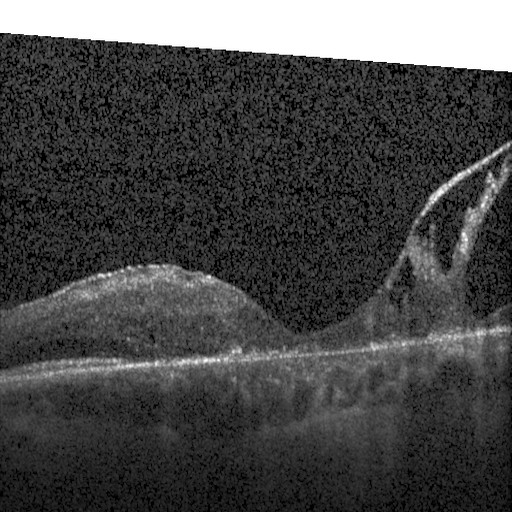
Optical coherence tomography scan, SD-OCT — Macular OCT: DME.